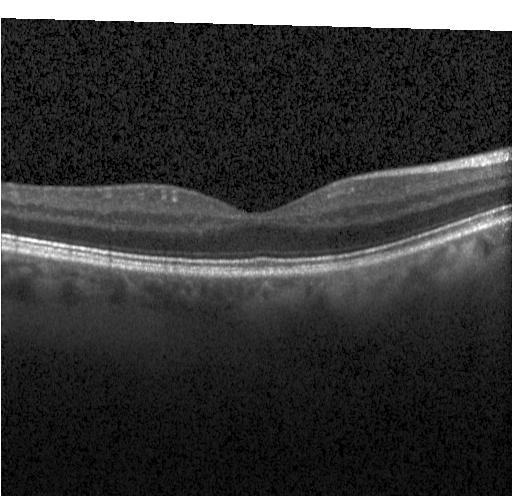

Dx: no evidence of choroidal neovascularization, diabetic macular edema, or drusen.